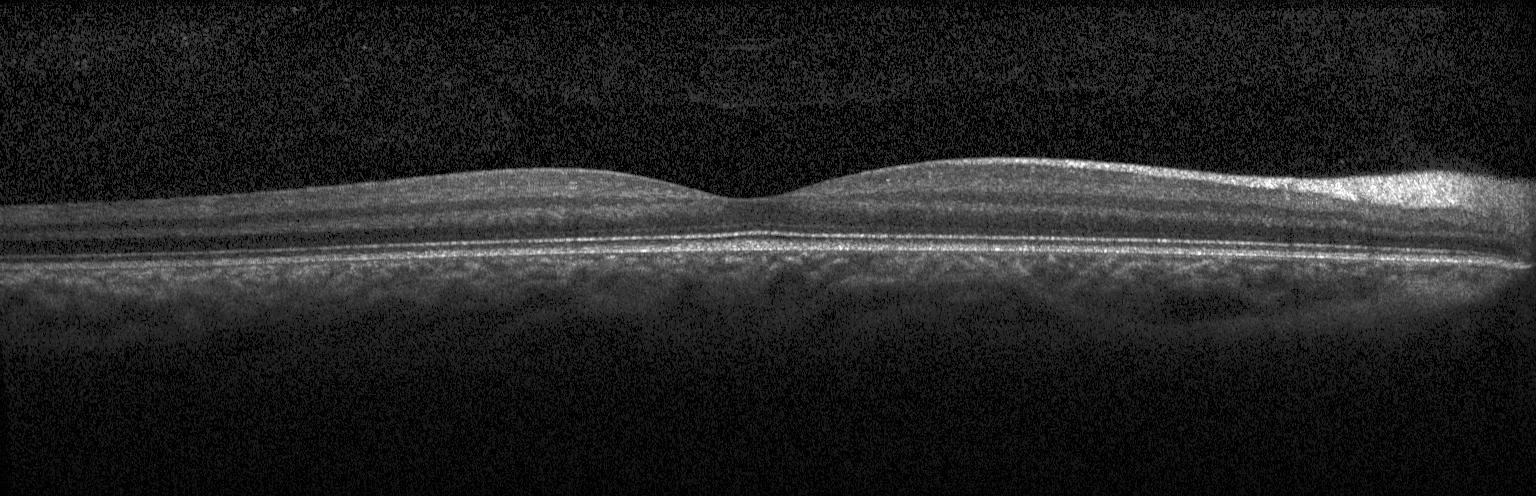

This B-scan demonstrates no CNV, DME, or drusen.